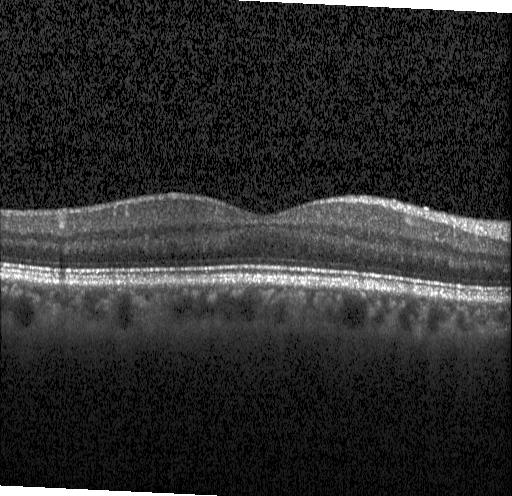

Retinal OCT cross-section. Fovea-centered. Spectral-domain optical coherence tomography. Heidelberg Spectralis — Diagnosis: no evidence of choroidal neovascularization, diabetic macular edema, or drusen.